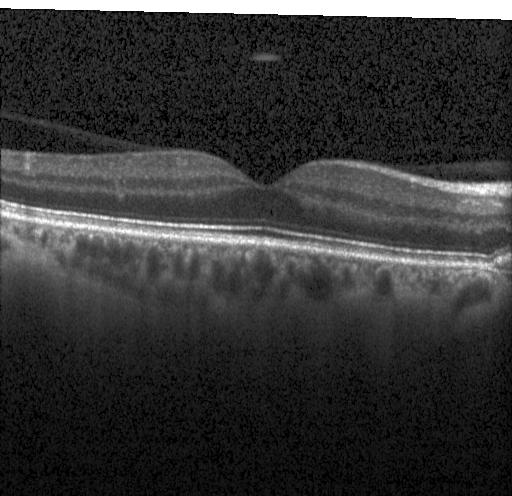 Retinal OCT B-scan.
Neither CNV, DME, nor drusen.